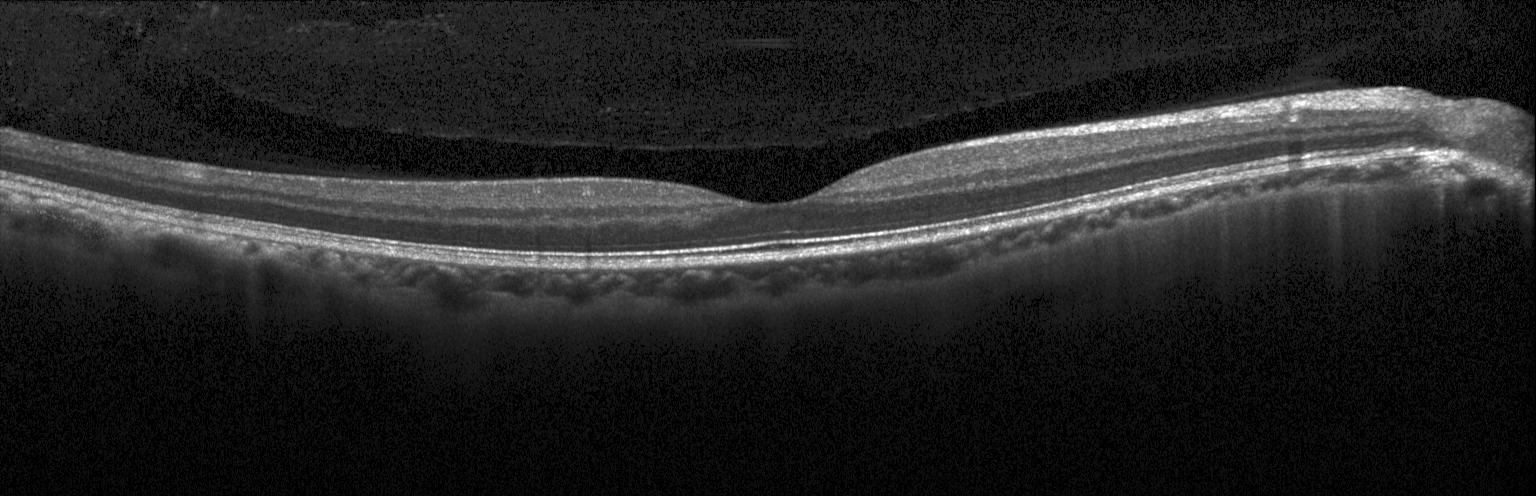 Acquired on a Heidelberg Spectralis; optical coherence tomography B-scan; spectral-domain optical coherence tomography; centered on the fovea
Assessment: no evidence of choroidal neovascularization, diabetic macular edema, or drusen.